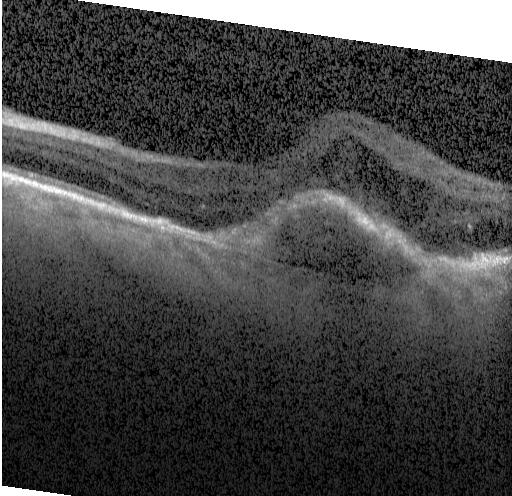
OCT finding: choroidal neovascularization (CNV).